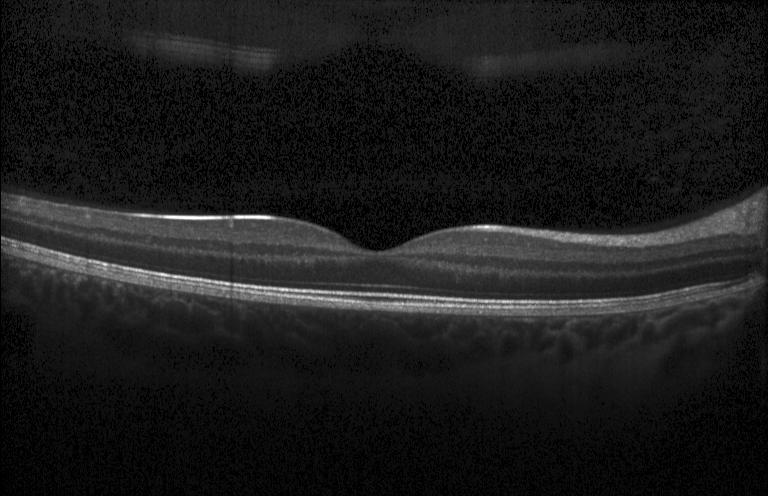

Spectral-domain OCT B-scan: no CNV, no DME, and no drusen.